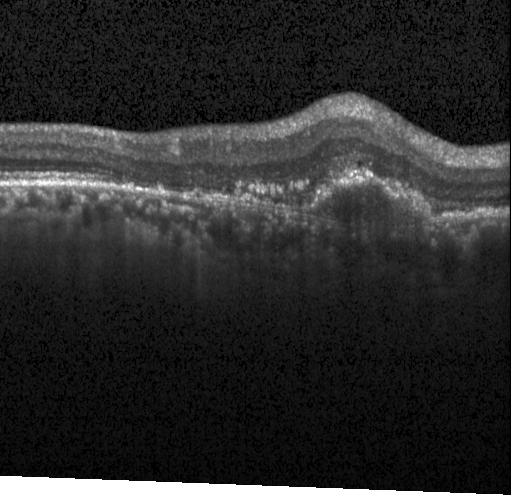 This B-scan demonstrates CNV.